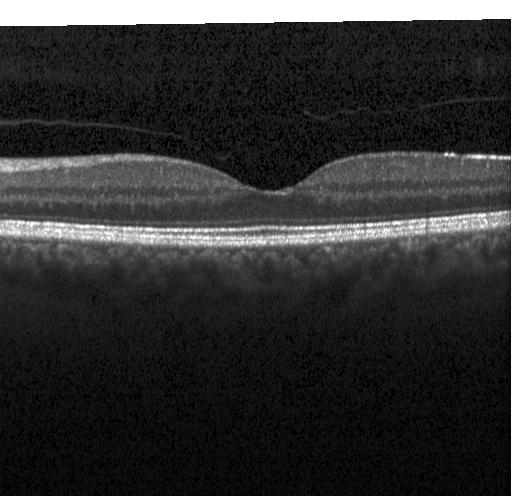

Spectral-domain OCT · retinal OCT B-scan · instrument: Heidelberg Spectralis · fovea-centered — Finding: no evidence of choroidal neovascularization, diabetic macular edema, or drusen.